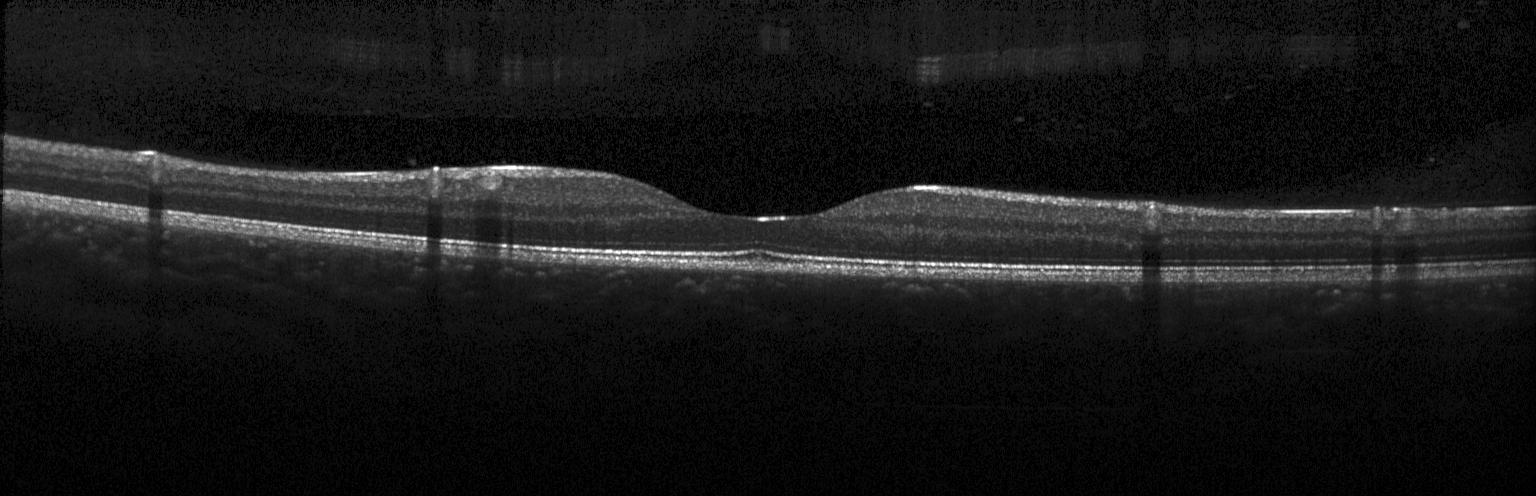
Macular OCT demonstrating no CNV, DME, or drusen.